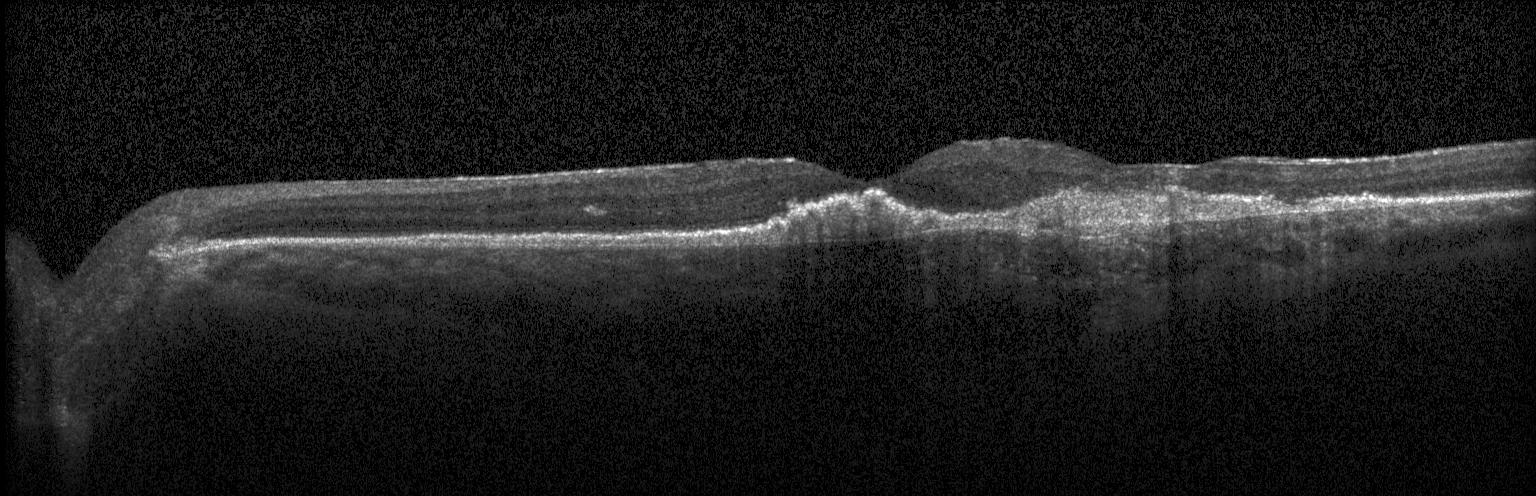

Acquired on a Heidelberg Spectralis. Retinal OCT cross-section. The scan shows a choroidal neovascular membrane.